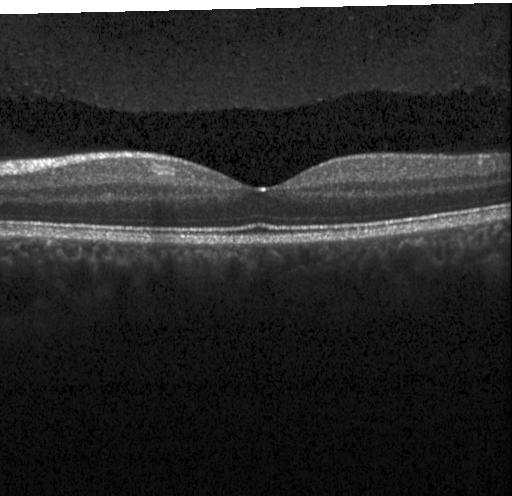 Retinal OCT B-scan.
OCT finding: no CNV, DME, or drusen.